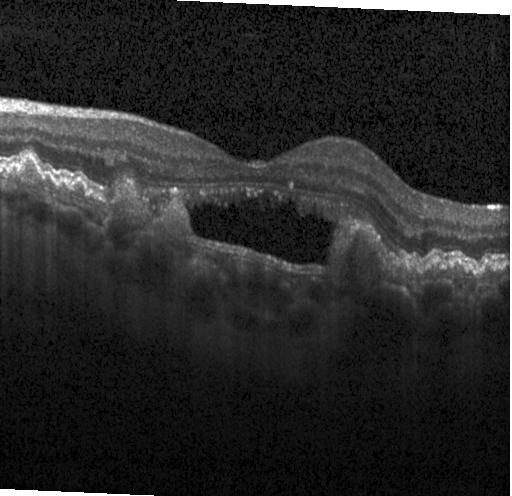

OCT line scan; spectral-domain optical coherence tomography
Assessment: a choroidal neovascular membrane.